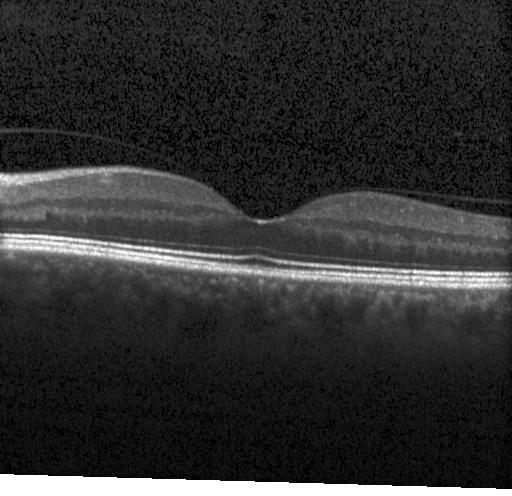
Finding: no choroidal neovascularization, diabetic macular edema, or drusen.